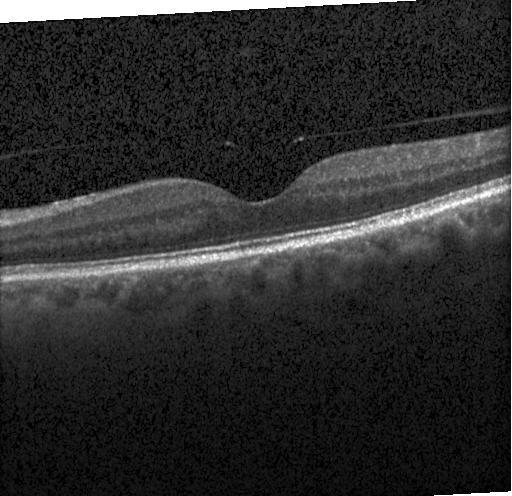

Retinal OCT cross-section; Heidelberg Spectralis.
Impression: no CNV, no DME, and no drusen.